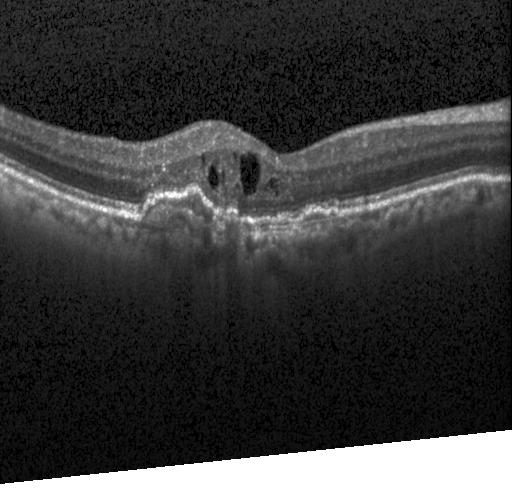 Retinal OCT cross-section showing a choroidal neovascular membrane.